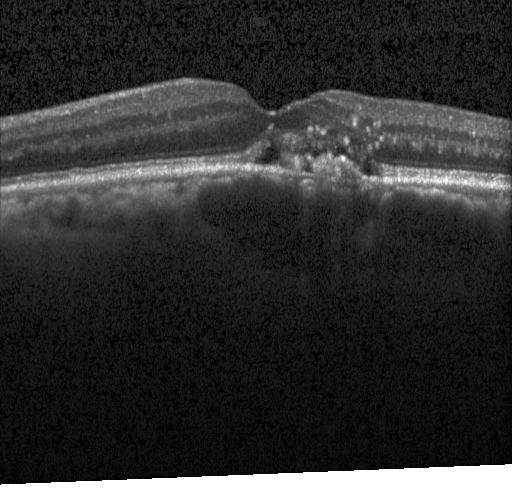 Dx: a choroidal neovascular membrane.